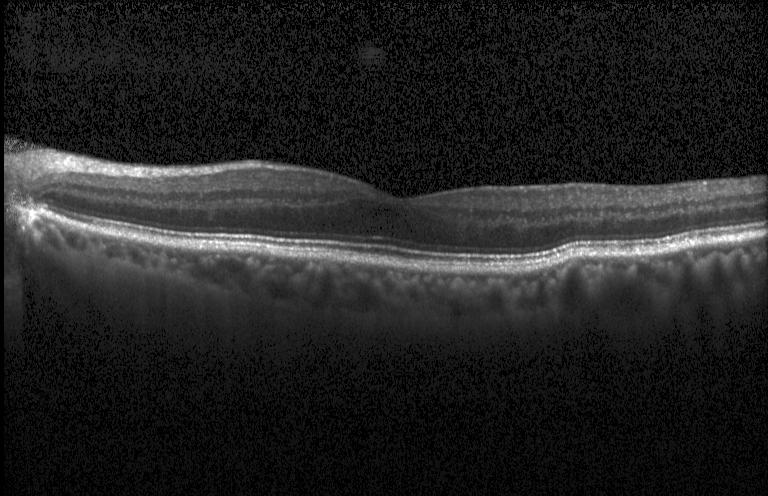

Impression: no evidence of CNV, DME, or drusen.